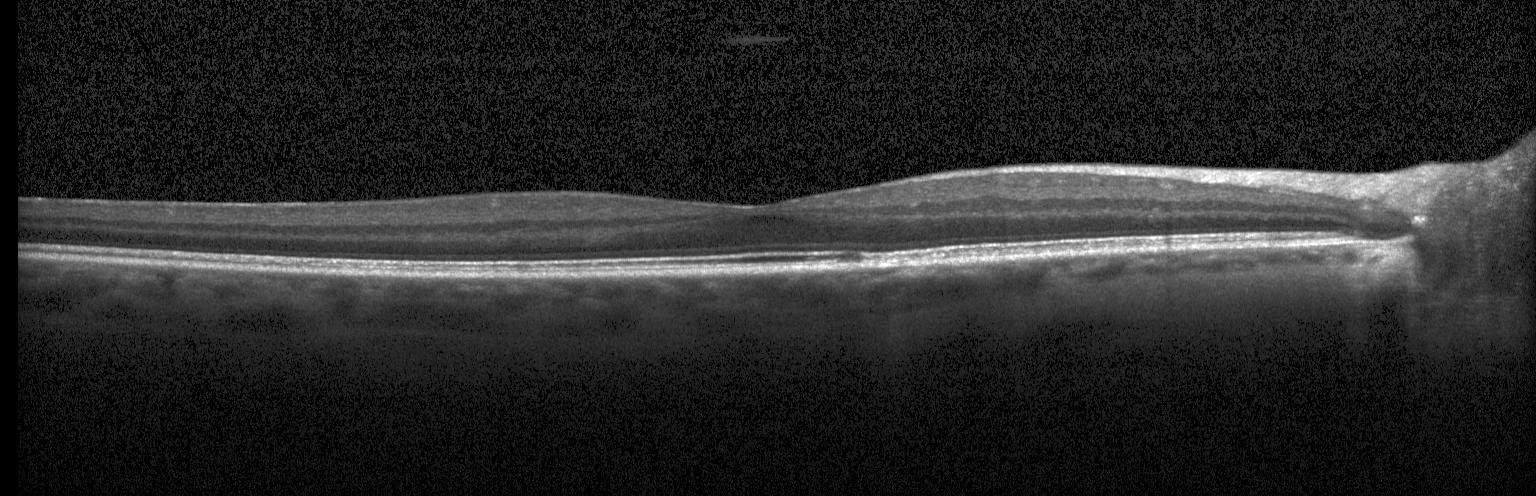 Optical coherence tomography B-scan, instrument: Heidelberg Spectralis — Assessment: neither choroidal neovascularization, diabetic macular edema, nor drusen.